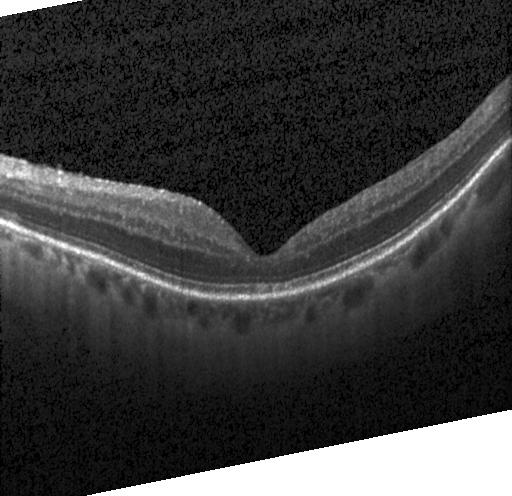 Macular OCT: no choroidal neovascularization, no diabetic macular edema, and no drusen.